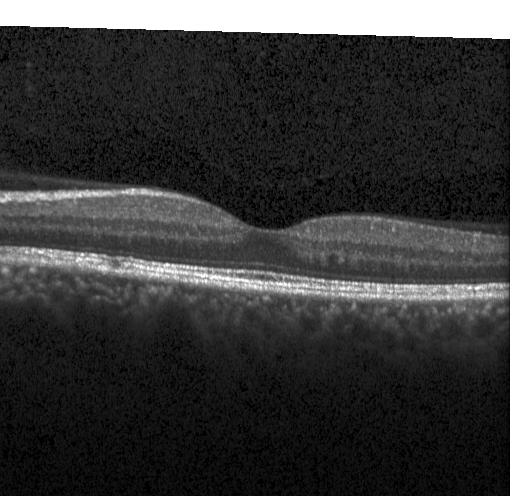 Macular OCT: no choroidal neovascularization, diabetic macular edema, or drusen.